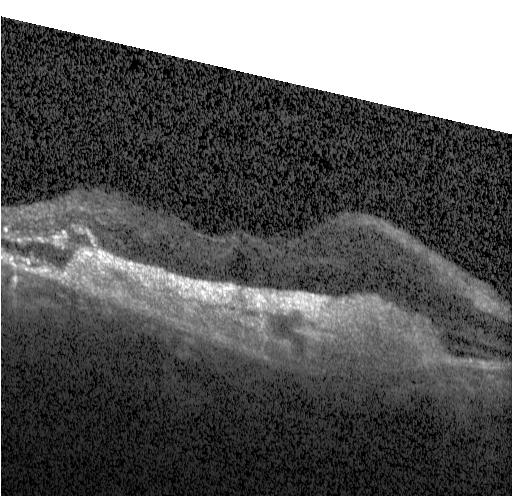 Macular scan; retinal OCT B-scan; SD-OCT; acquired on a Heidelberg Spectralis. Finding: CNV.